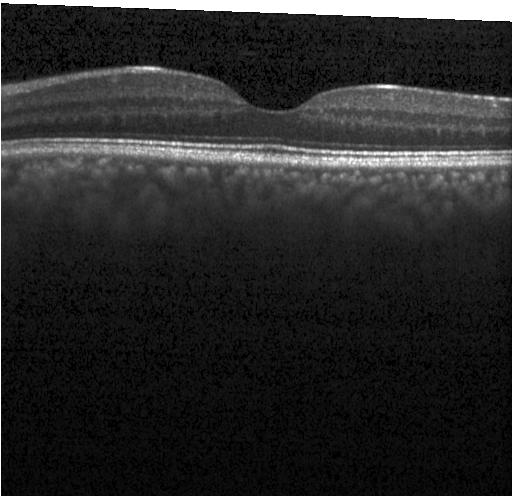
Dx: no evidence of choroidal neovascularization, diabetic macular edema, or drusen.